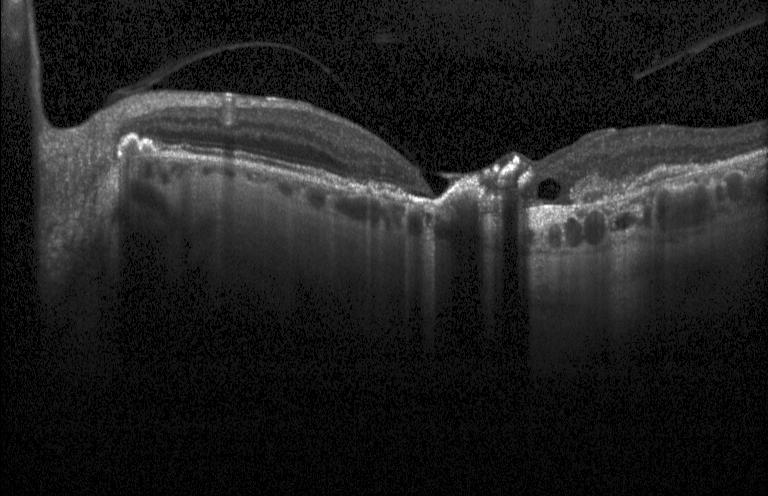 OCT line scan
Dx: choroidal neovascularization (CNV).